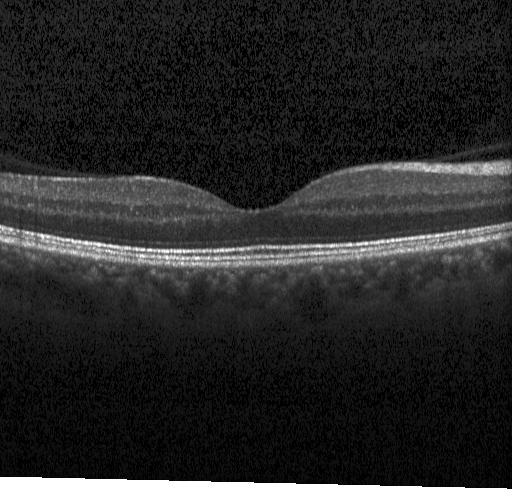
OCT finding: no choroidal neovascularization, diabetic macular edema, or drusen.